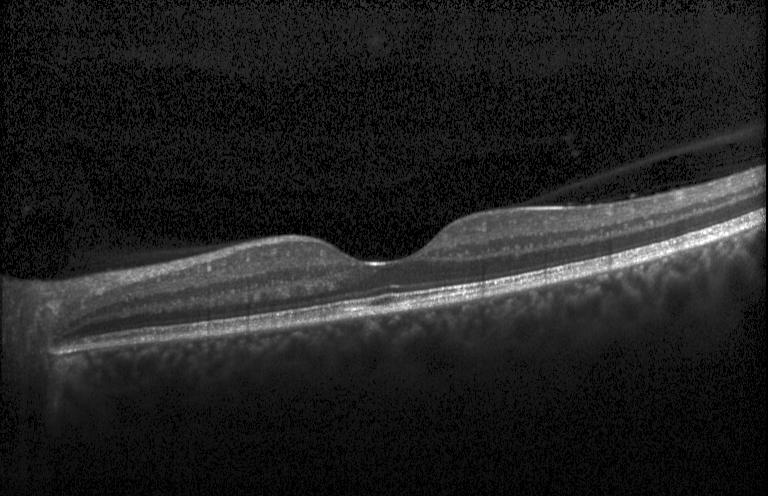
Macular OCT: no choroidal neovascularization, diabetic macular edema, or drusen.